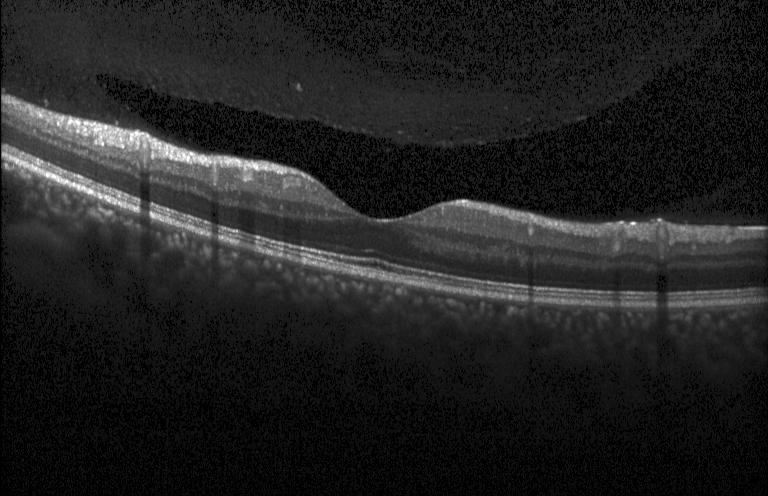 Macular OCT demonstrating no evidence of choroidal neovascularization, diabetic macular edema, or drusen.